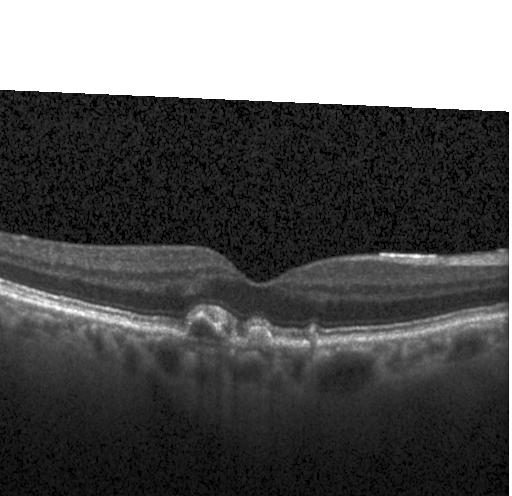
Macular OCT: a choroidal neovascular membrane.